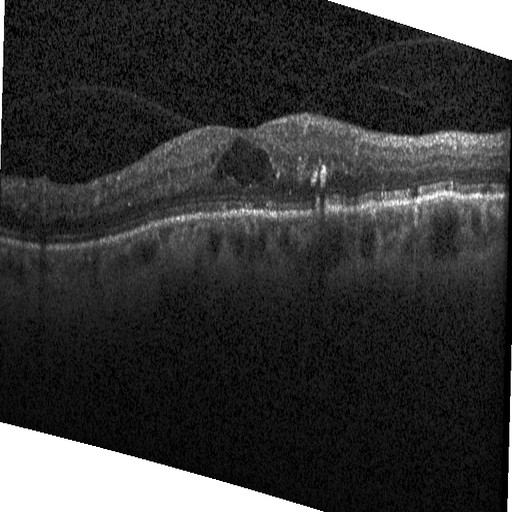

Diagnosis: diabetic macular edema.